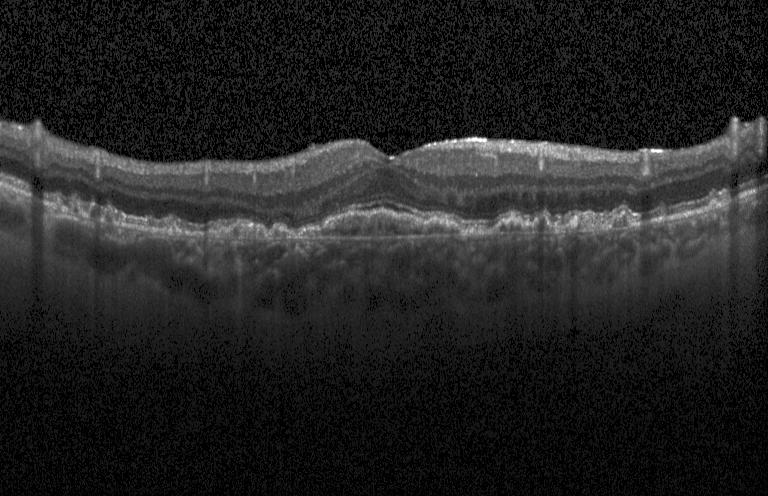

Centered on the fovea; optical coherence tomography scan; SD-OCT. OCT finding: a choroidal neovascular membrane.